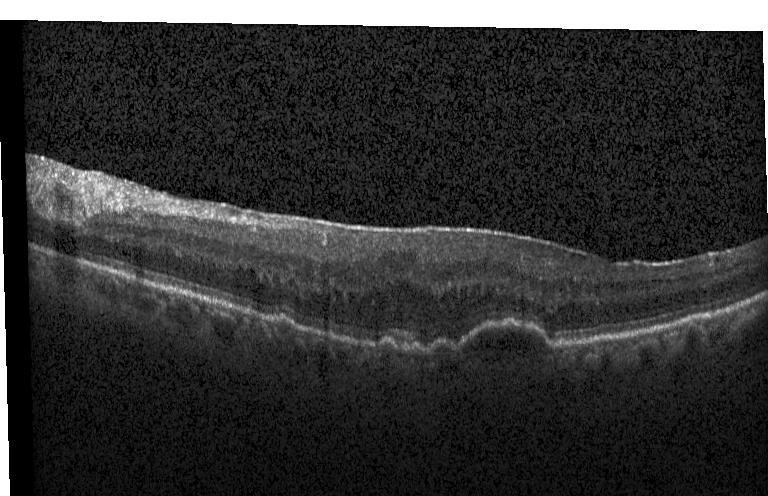 Optical coherence tomography scan · acquired on a Heidelberg Spectralis · spectral-domain optical coherence tomography. Macular OCT: a choroidal neovascular membrane.